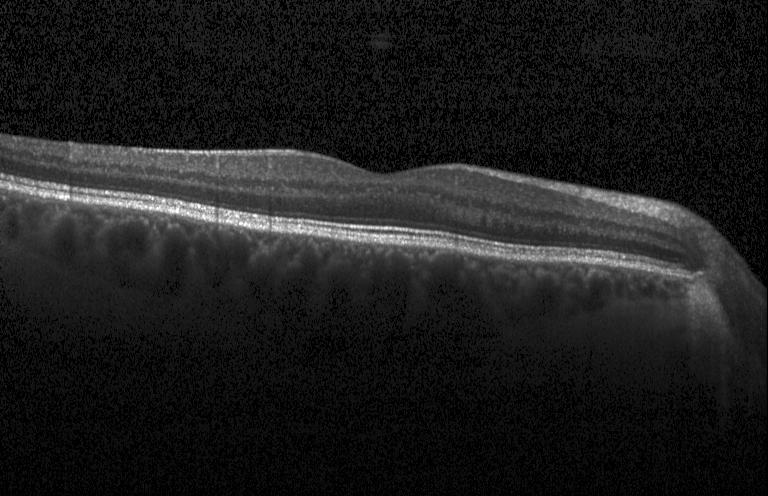 Acquired on a Heidelberg Spectralis, spectral-domain OCT, retinal OCT cross-section, centered on the fovea
Diagnosis: neither CNV, DME, nor drusen.